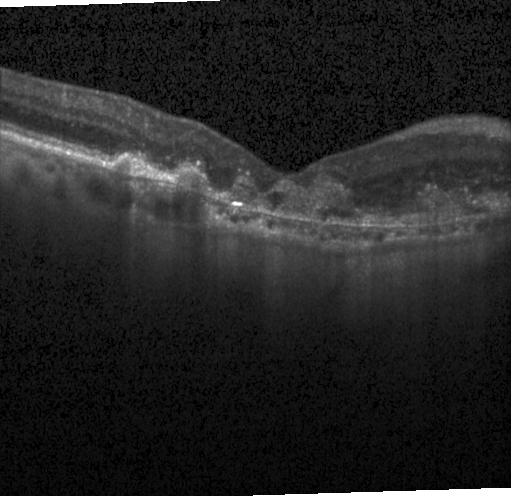

OCT scan showing a choroidal neovascular membrane.